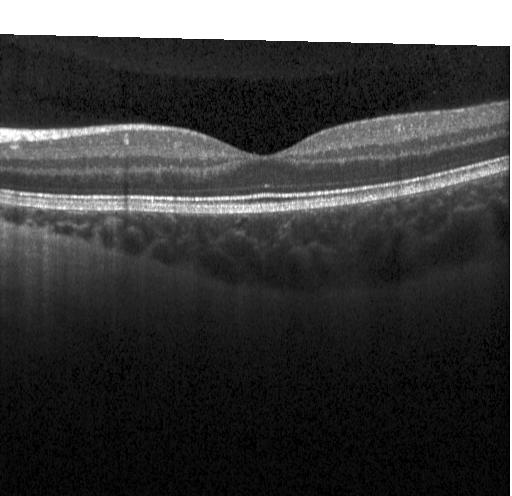 OCT line scan. Horizontal scan through the fovea. Heidelberg Spectralis OCT system. Spectral-domain optical coherence tomography.
Finding: neither choroidal neovascularization, diabetic macular edema, nor drusen.